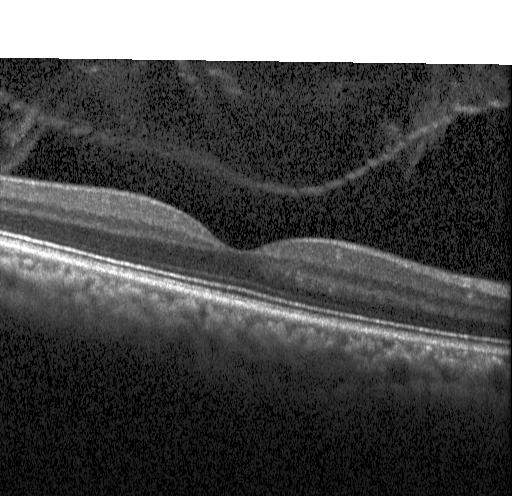 OCT scan showing no CNV, DME, or drusen.